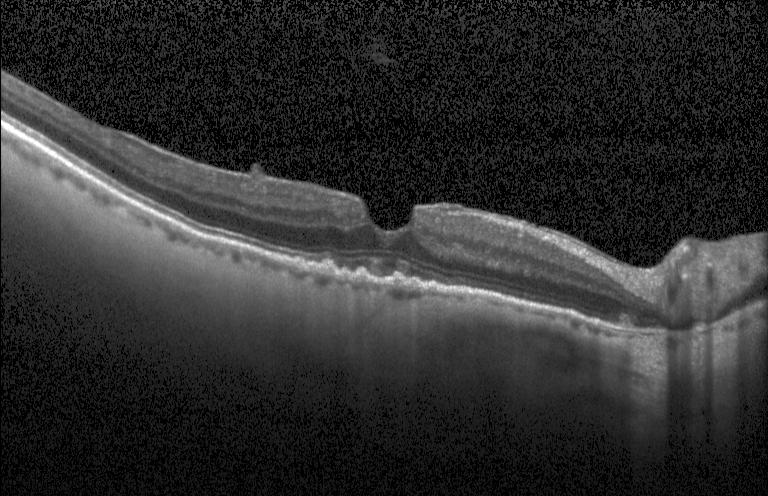 The scan shows sub-RPE drusenoid deposits.